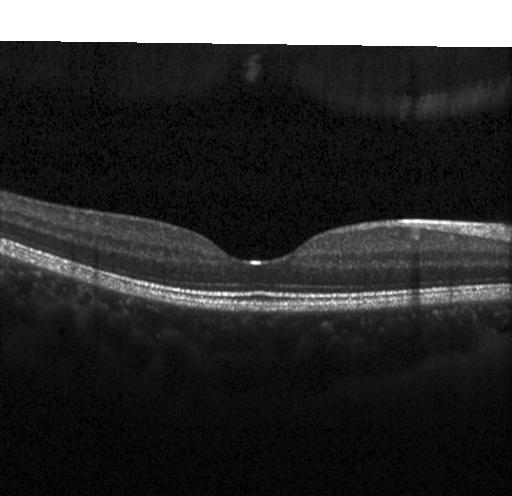

Optical coherence tomography scan. OCT finding: no choroidal neovascularization, diabetic macular edema, or drusen.